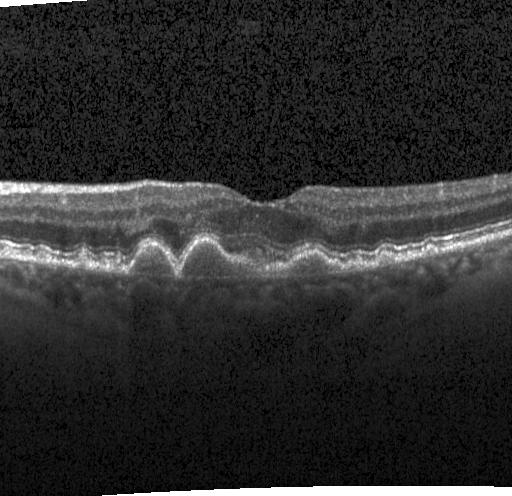
Optical coherence tomography B-scan; spectral-domain optical coherence tomography.
Finding: a choroidal neovascular membrane.